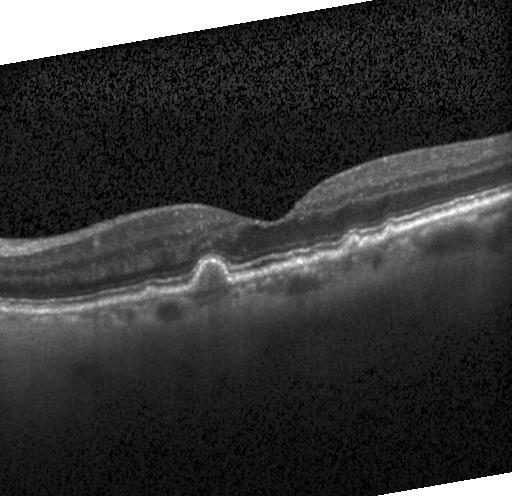
Spectral-domain OCT; retinal OCT B-scan; Heidelberg Spectralis OCT system.
Macular OCT: drusen.